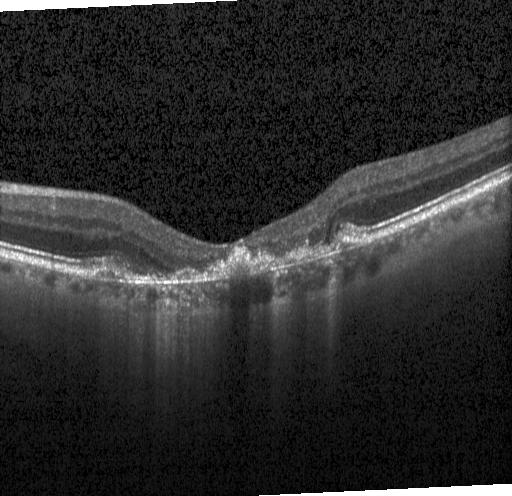
The scan shows CNV.